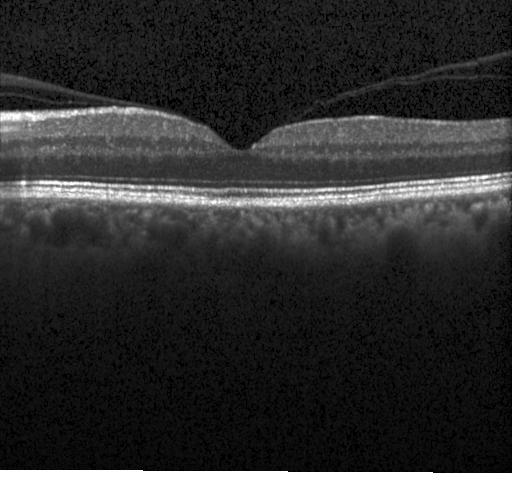

OCT B-scan. Spectral-domain optical coherence tomography. Heidelberg Spectralis OCT system.
Impression: no CNV, DME, or drusen.